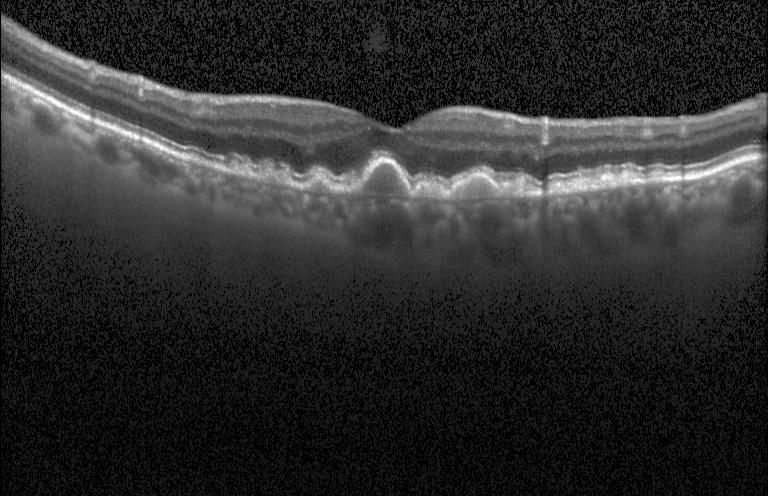 The scan shows multiple drusen.